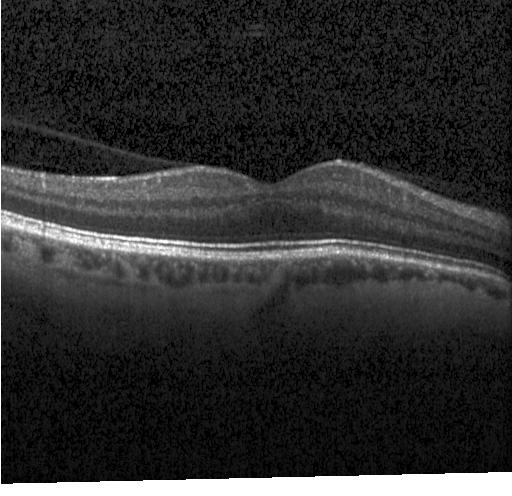

This B-scan demonstrates neither CNV, DME, nor drusen.